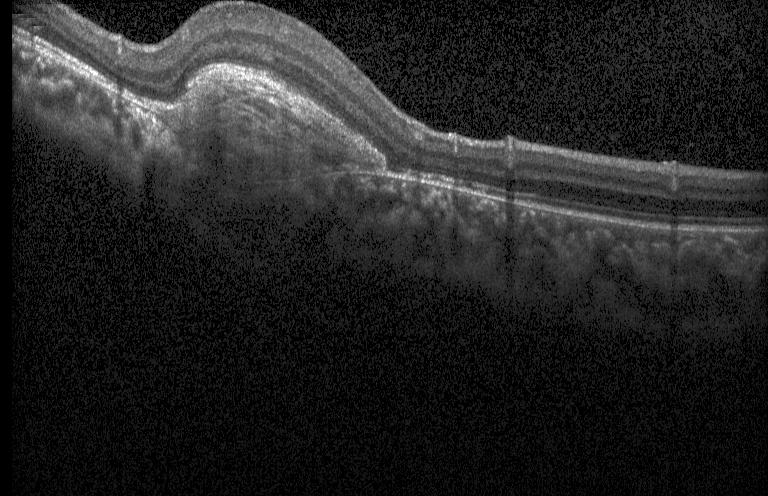

Dx: a choroidal neovascular membrane.